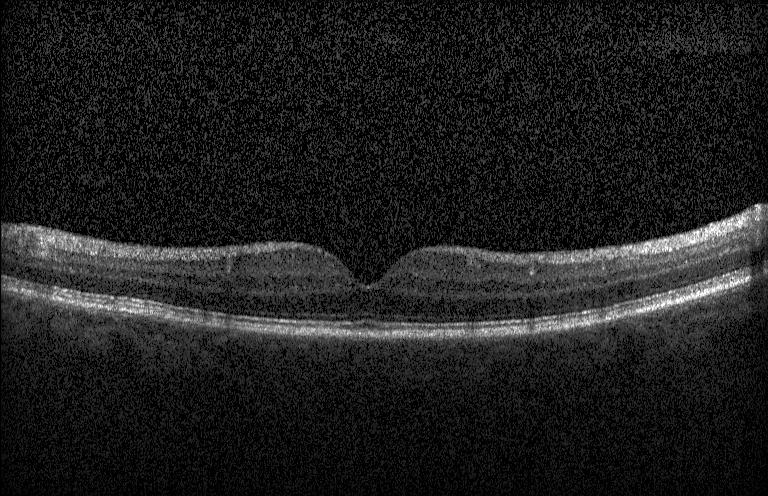

OCT finding: no evidence of choroidal neovascularization, diabetic macular edema, or drusen.